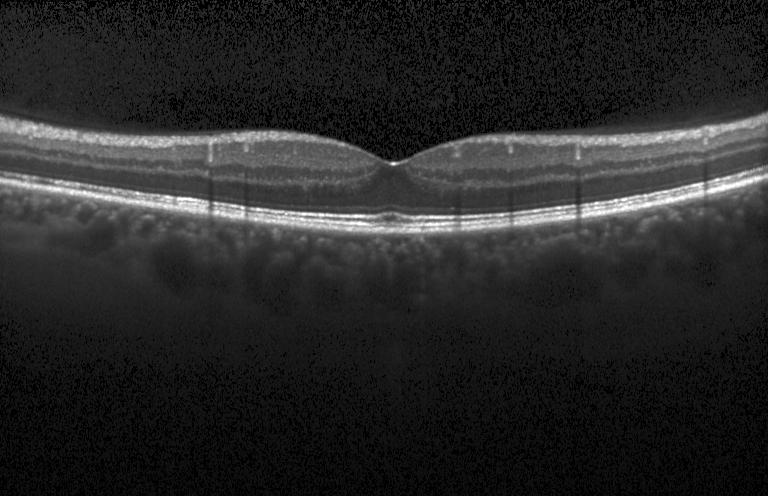 Acquired on a Heidelberg Spectralis. OCT B-scan — The scan shows no choroidal neovascularization, diabetic macular edema, or drusen.